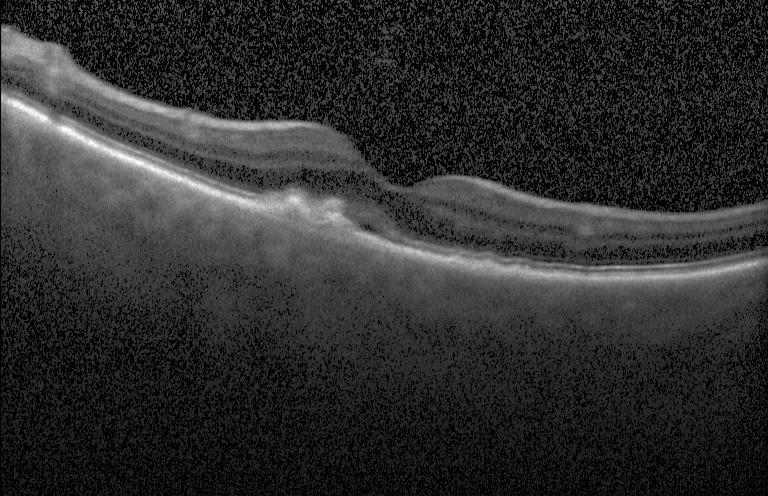 OCT B-scan showing CNV.